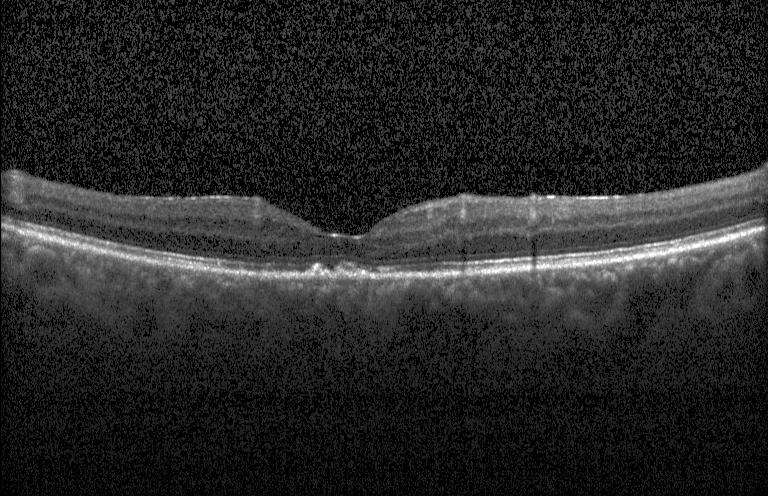 Optical coherence tomography B-scan · acquired on a Heidelberg Spectralis · horizontal scan through the fovea. Diagnosis: multiple drusen.